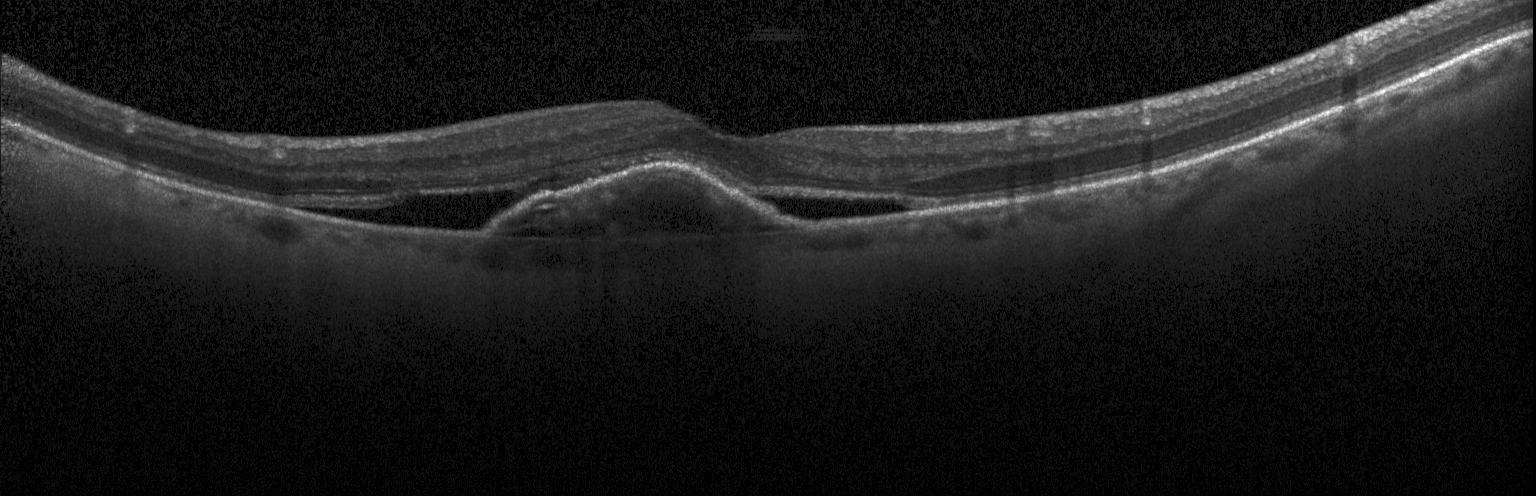

Heidelberg Spectralis OCT system. OCT B-scan.
Choroidal neovascularization.